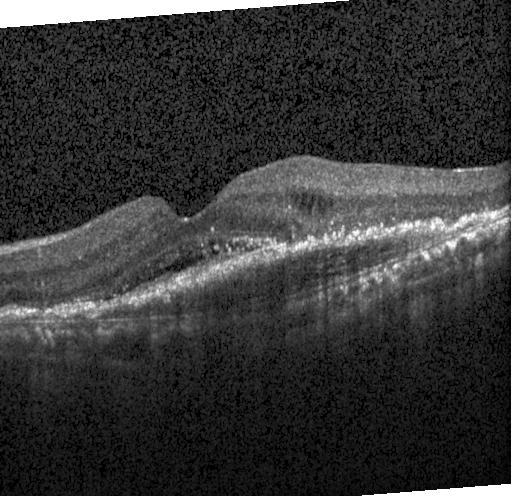

Optical coherence tomography scan, SD-OCT, fovea-centered — Assessment: a choroidal neovascular membrane.